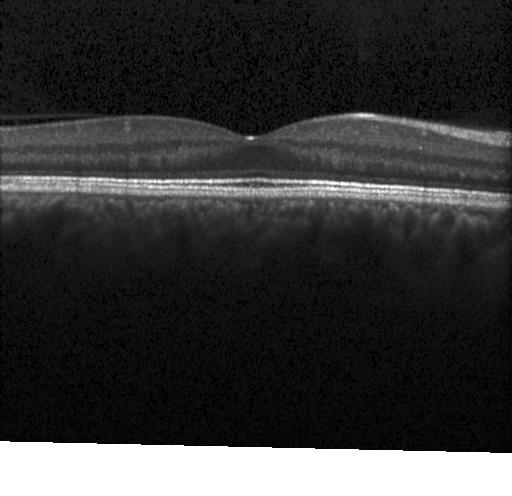

Through the macula. Heidelberg Spectralis OCT system. Spectral-domain OCT. Retinal OCT B-scan
Assessment: no choroidal neovascularization, diabetic macular edema, or drusen.